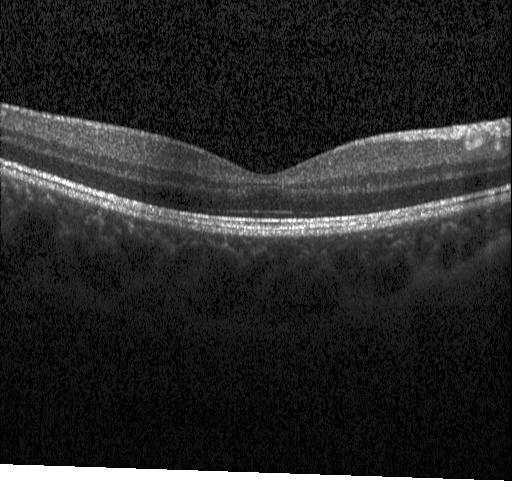

OCT line scan; SD-OCT.
Diagnosis: no CNV, DME, or drusen.